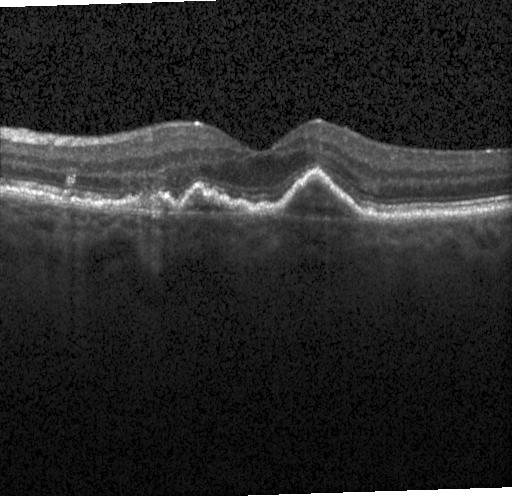

CNV.